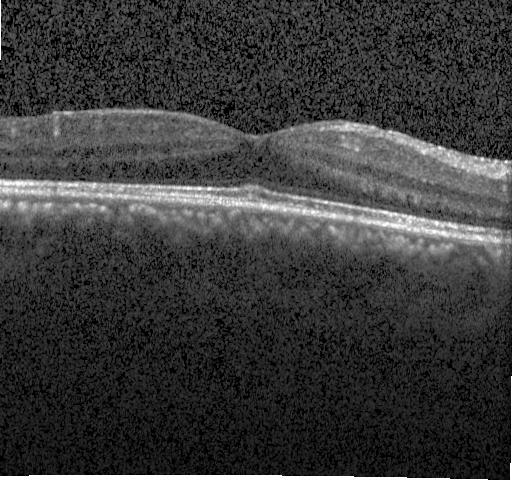 Dx: neither choroidal neovascularization, diabetic macular edema, nor drusen.